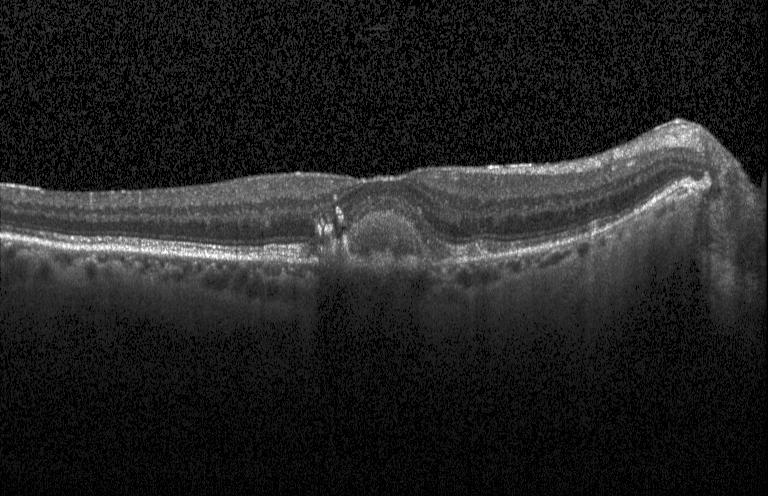 SD-OCT; Heidelberg Spectralis; horizontal scan through the fovea; retinal OCT cross-section. This B-scan demonstrates a choroidal neovascular membrane.